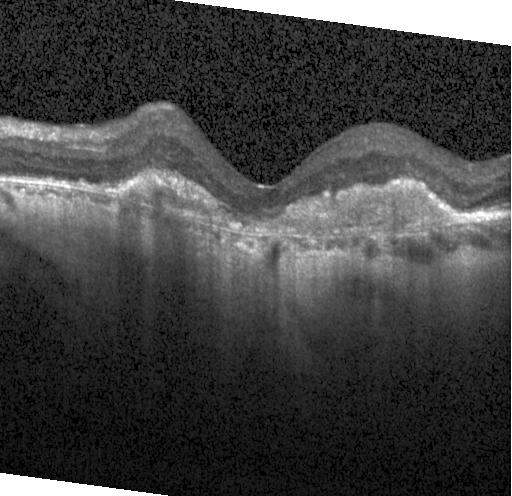
Spectral-domain optical coherence tomography, acquired on a Heidelberg Spectralis, centered on the fovea, optical coherence tomography B-scan — Assessment: choroidal neovascularization.